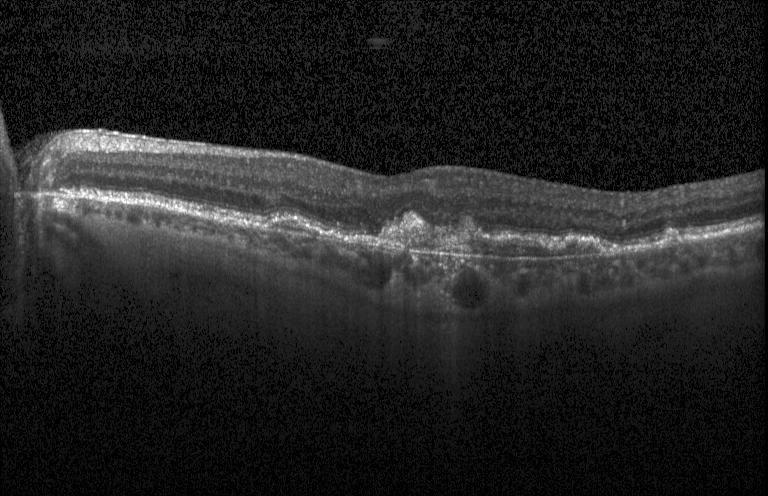 Optical coherence tomography scan, spectral-domain OCT, instrument: Heidelberg Spectralis
Choroidal neovascularization.